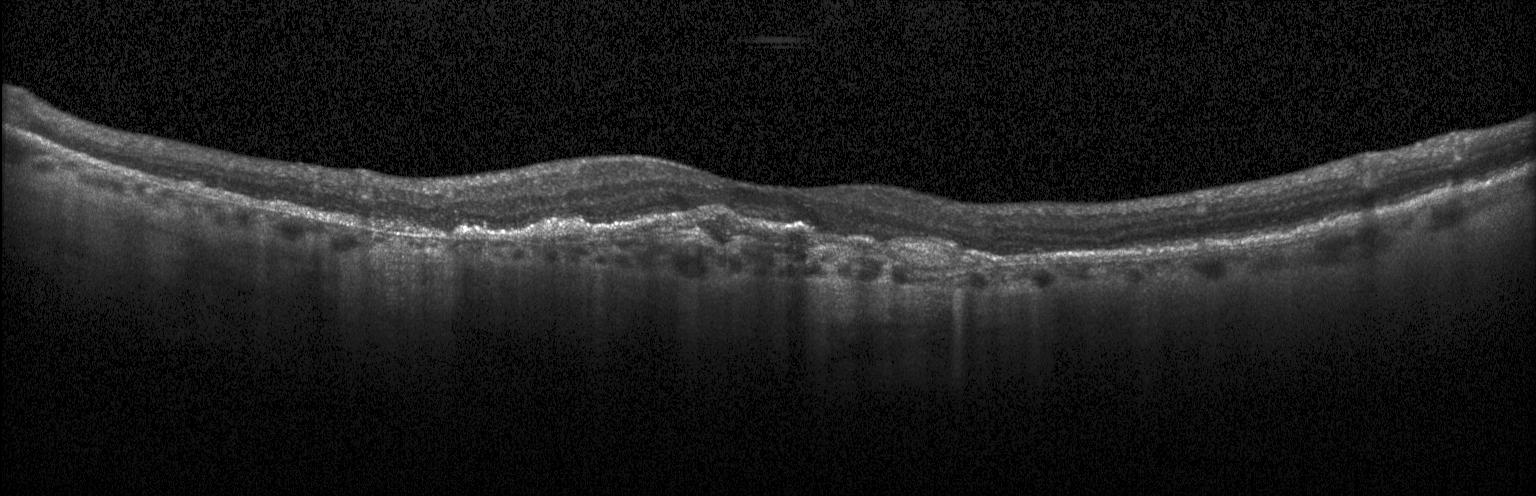 Macular scan · OCT B-scan · acquired on a Heidelberg Spectralis — Diagnosis: choroidal neovascularization (CNV).